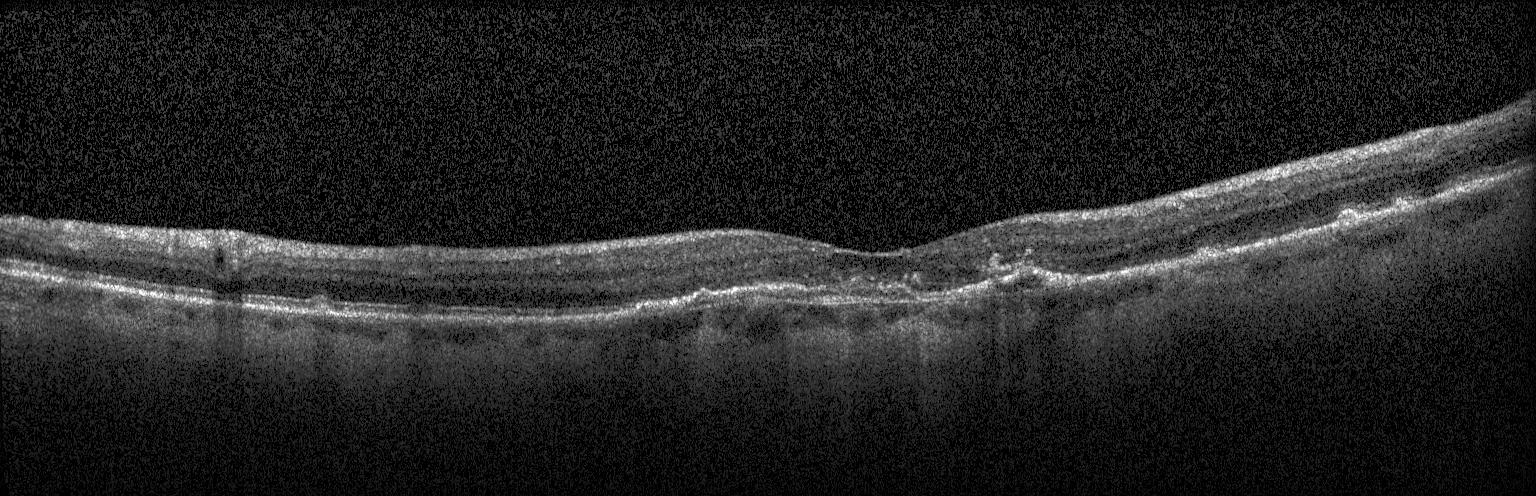

OCT finding: a choroidal neovascular membrane.